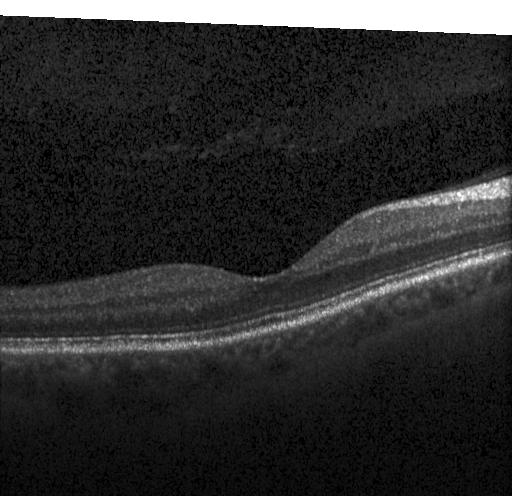
Acquired on a Heidelberg Spectralis; macular scan; spectral-domain optical coherence tomography; OCT B-scan — Macular OCT: no evidence of choroidal neovascularization, diabetic macular edema, or drusen.